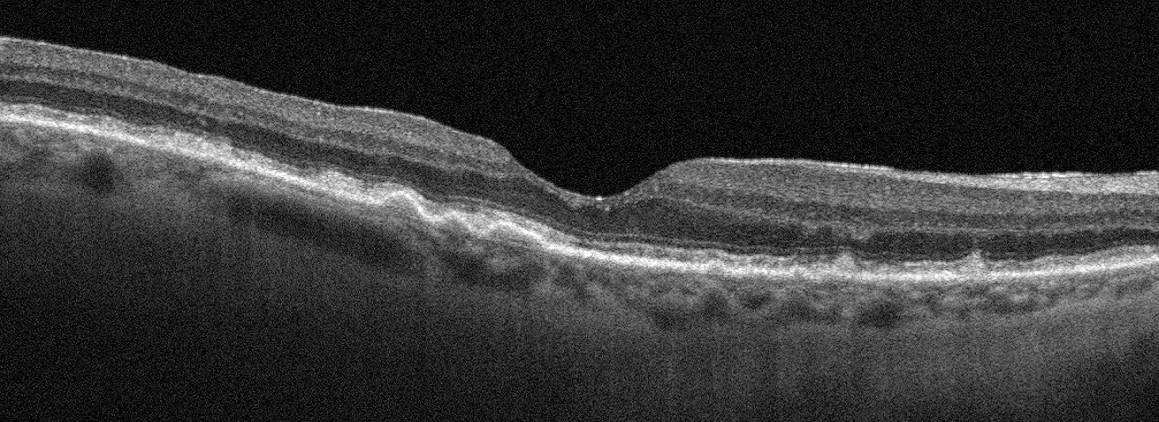 Instrument: Optovue Avanti RTVue XR, OD, retinal OCT cross-section, macular scan.
OCT finding: age-related macular degeneration.